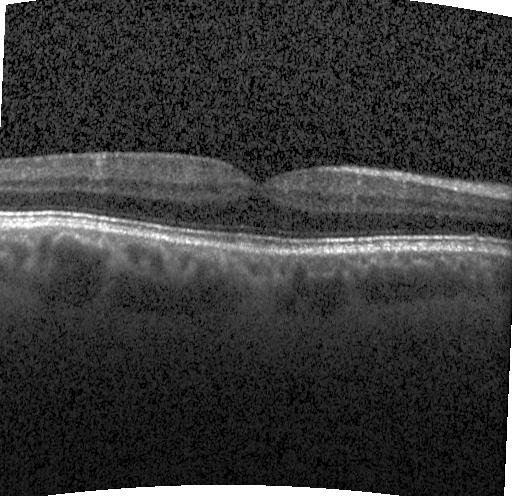 Centered on the fovea, OCT B-scan, spectral-domain optical coherence tomography
The scan shows no CNV, no DME, and no drusen.